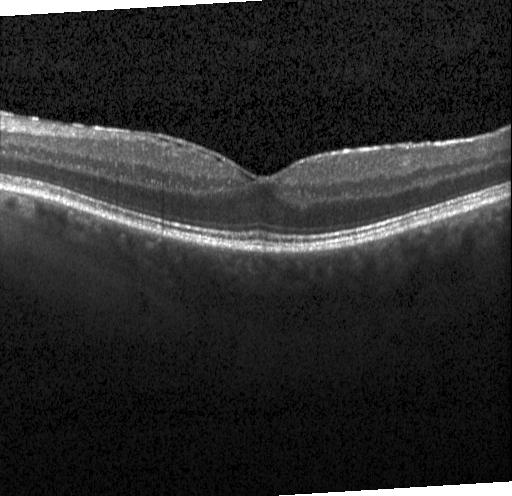 Macular OCT: neither choroidal neovascularization, diabetic macular edema, nor drusen.